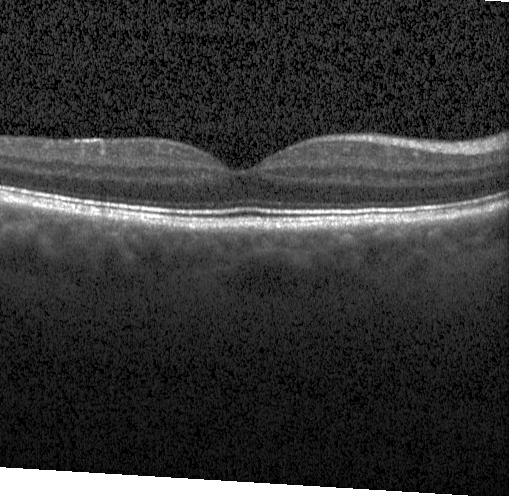
SD-OCT. OCT B-scan. Through the macula
Impression: no choroidal neovascularization, diabetic macular edema, or drusen.